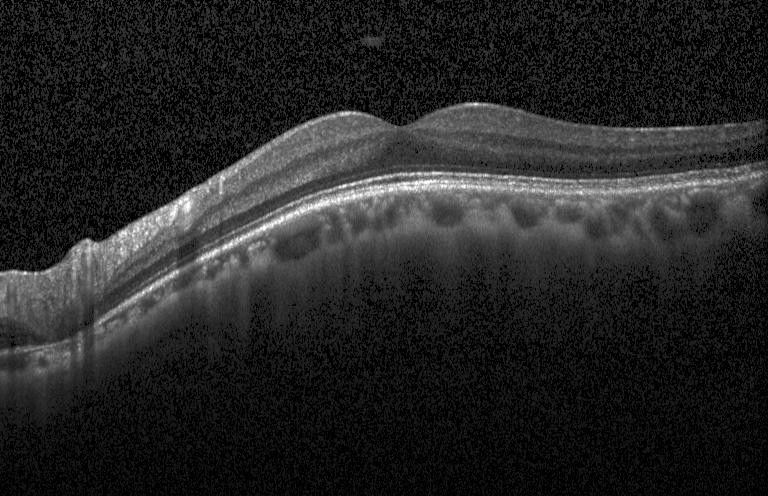 Retinal OCT cross-section; macular scan; spectral-domain OCT. The scan shows no choroidal neovascularization, no diabetic macular edema, and no drusen.